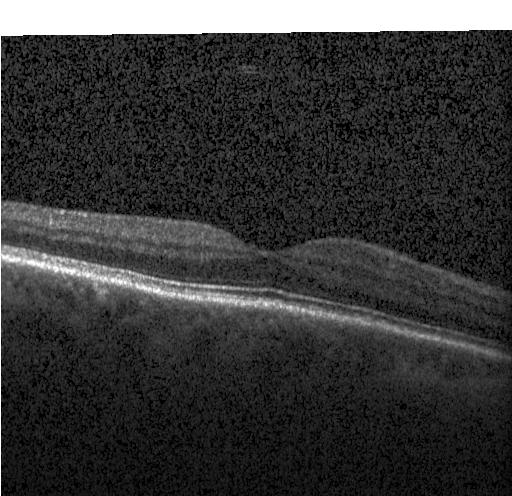 Optical coherence tomography scan · instrument: Heidelberg Spectralis · through the macula.
Impression: no evidence of CNV, DME, or drusen.